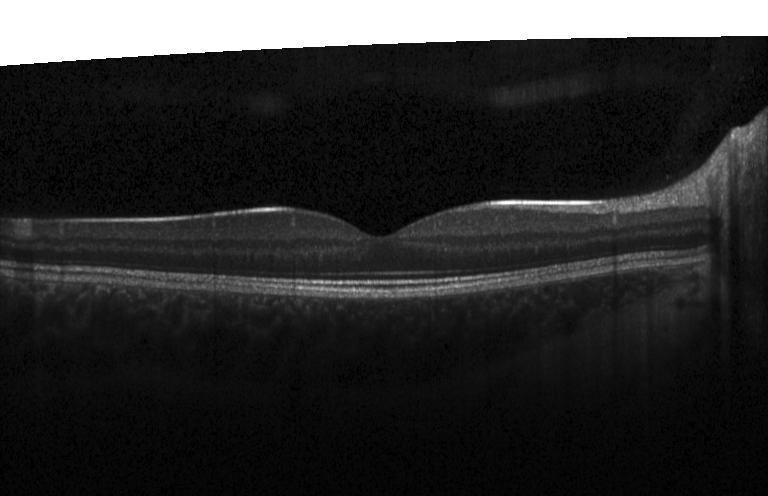

Impression: no CNV, no DME, and no drusen.